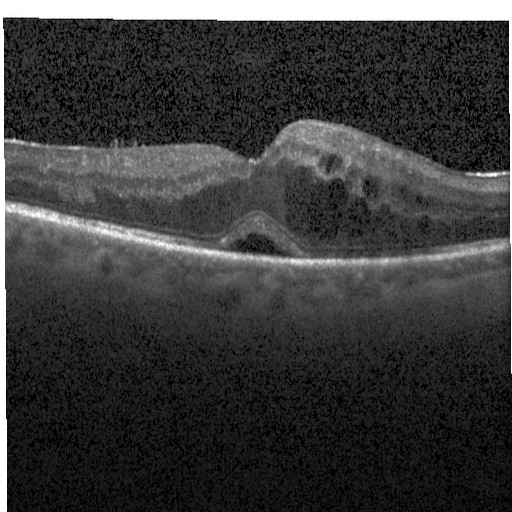
Impression: diabetic macular edema.